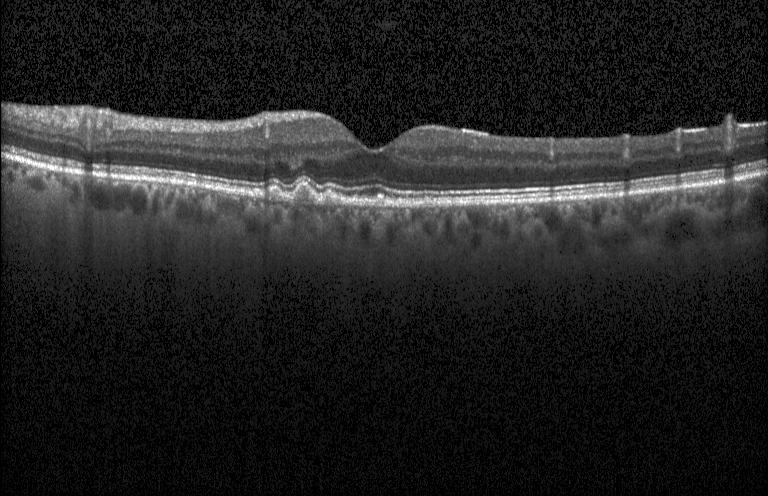
OCT B-scan. OCT finding: drusen.